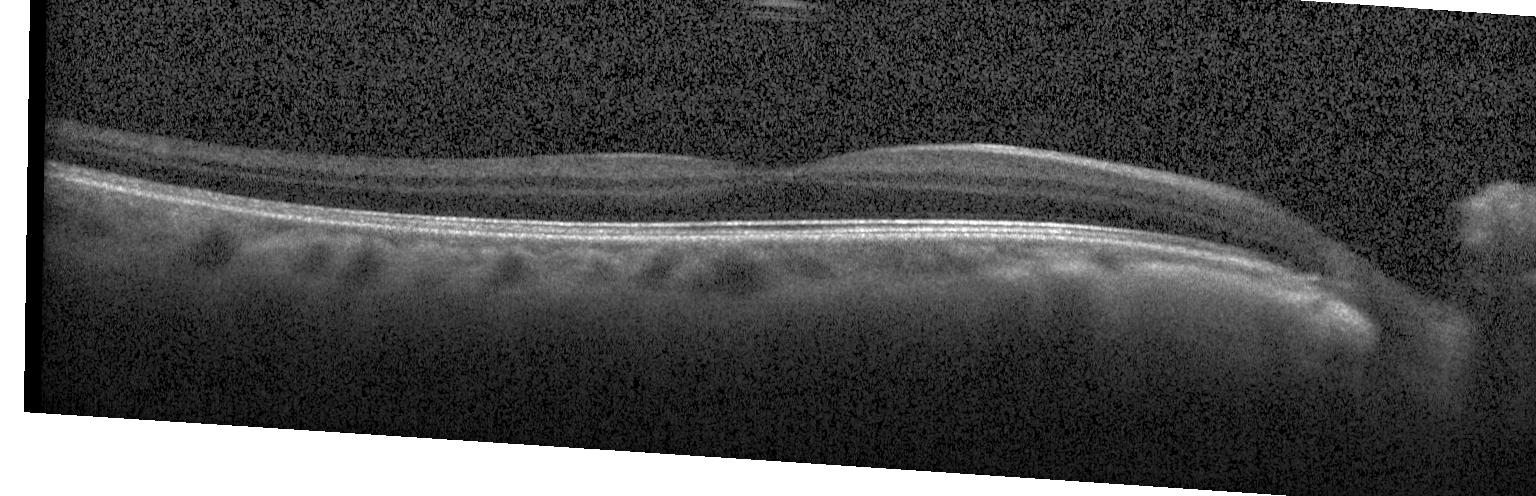 Macular OCT: no choroidal neovascularization, diabetic macular edema, or drusen.